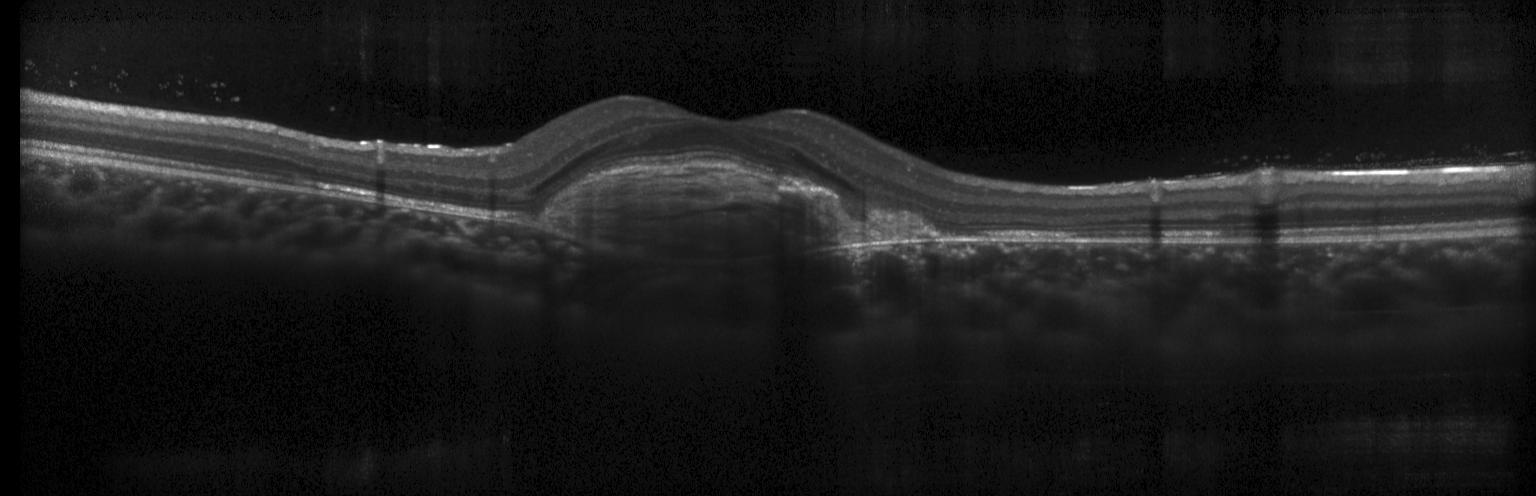 Diagnosis: a choroidal neovascular membrane.